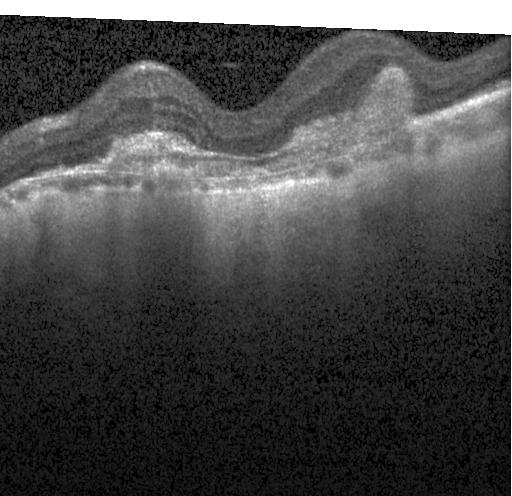 OCT B-scan
Impression: a choroidal neovascular membrane.